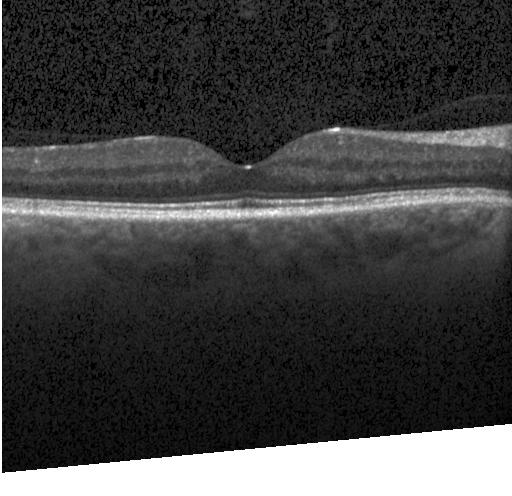 Optical coherence tomography scan; acquired on a Heidelberg Spectralis
Diagnosis: no evidence of choroidal neovascularization, diabetic macular edema, or drusen.